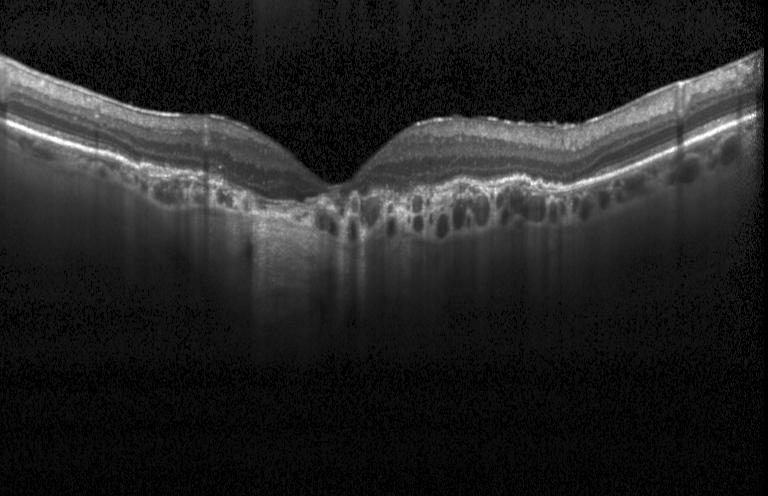
Assessment: a choroidal neovascular membrane.